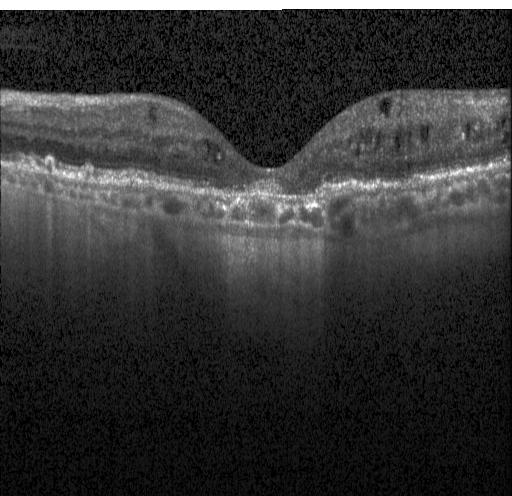

Acquired on a Heidelberg Spectralis. OCT line scan.
Diagnosis: a choroidal neovascular membrane.